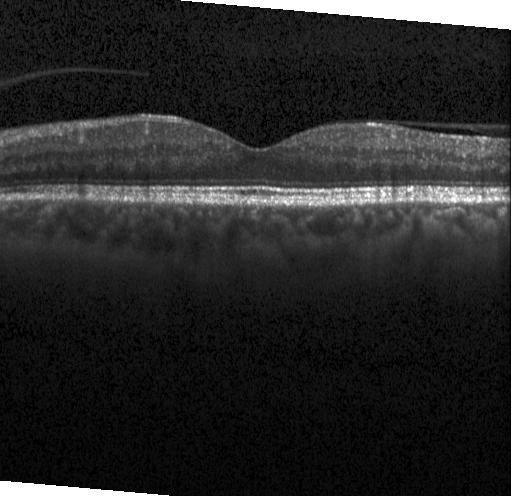 Heidelberg Spectralis OCT system · retinal OCT cross-section · SD-OCT. Diagnosis: no choroidal neovascularization, no diabetic macular edema, and no drusen.